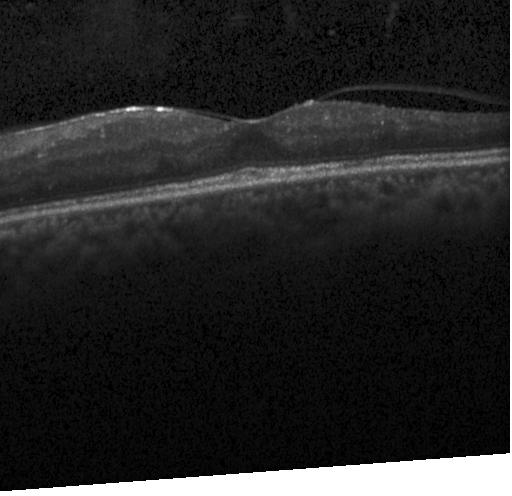 Optical coherence tomography scan; Heidelberg Spectralis
Diabetic macular edema (DME).